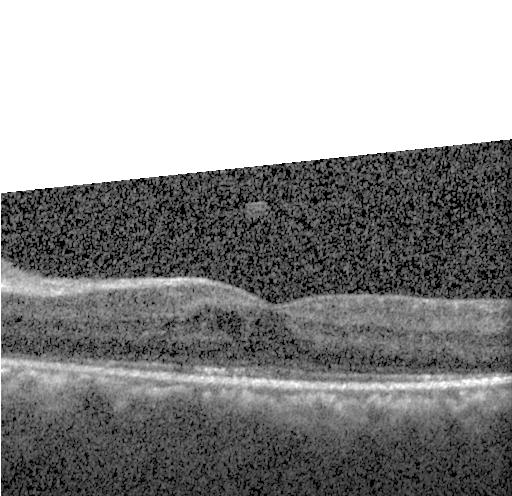
Through the macula, OCT line scan.
Diagnosis: diabetic macular edema.